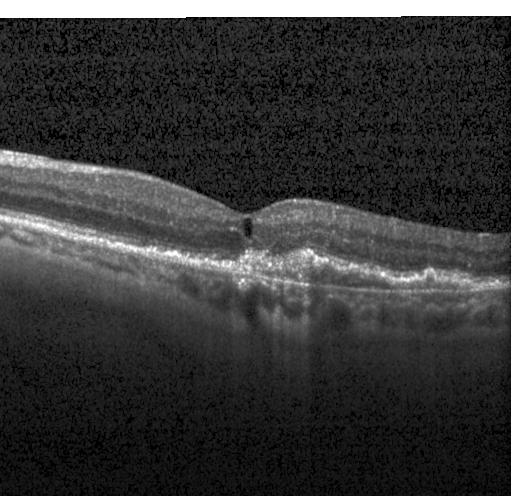

Optical coherence tomography B-scan; SD-OCT; instrument: Heidelberg Spectralis. Impression: CNV.